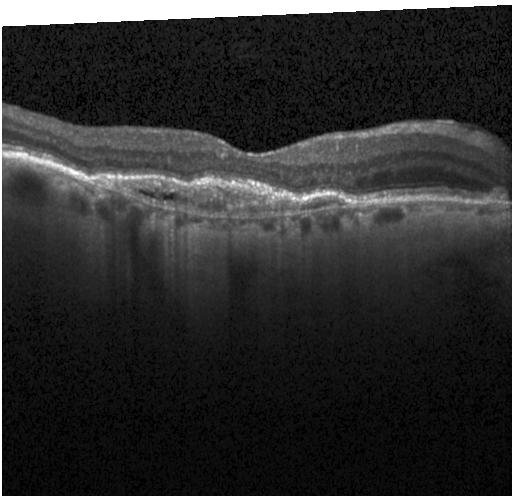
Macular OCT demonstrating a choroidal neovascular membrane.